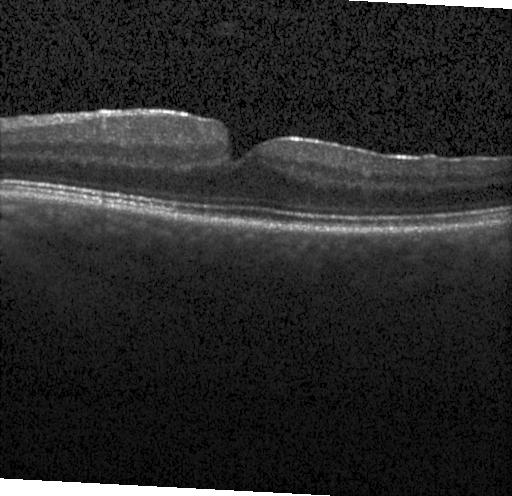
Impression: neither choroidal neovascularization, diabetic macular edema, nor drusen.